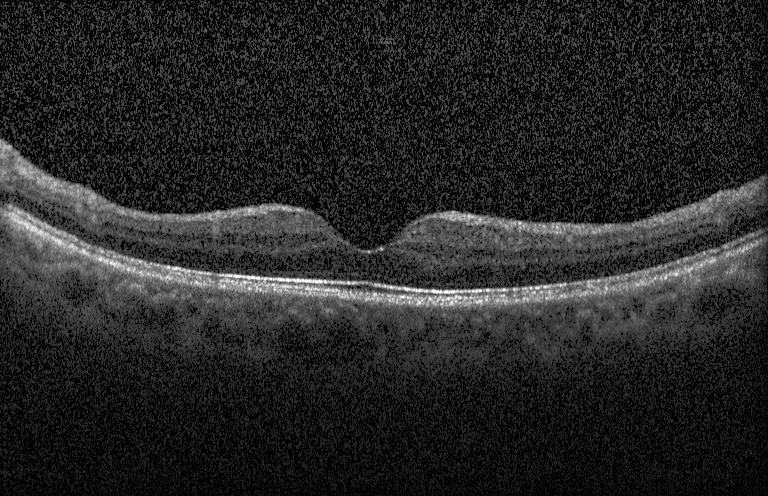
Finding: no choroidal neovascularization, no diabetic macular edema, and no drusen.